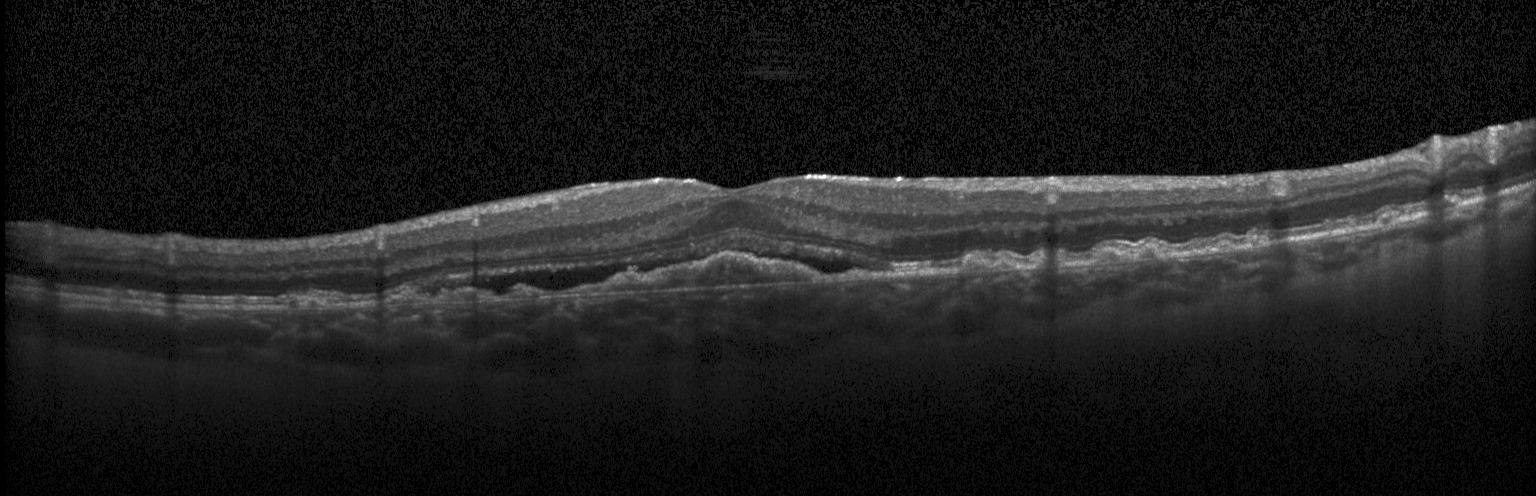

Choroidal neovascularization (CNV).